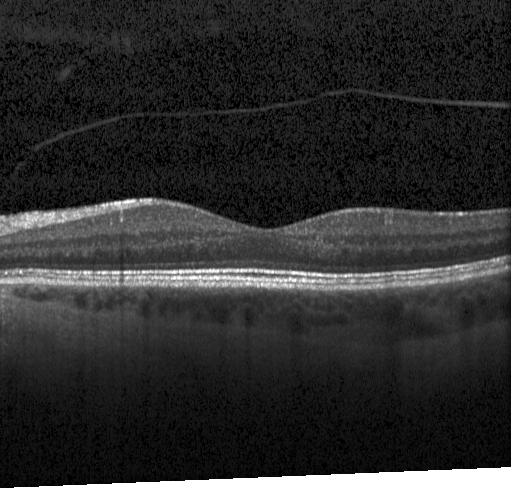

Spectral-domain OCT B-scan: neither CNV, DME, nor drusen.